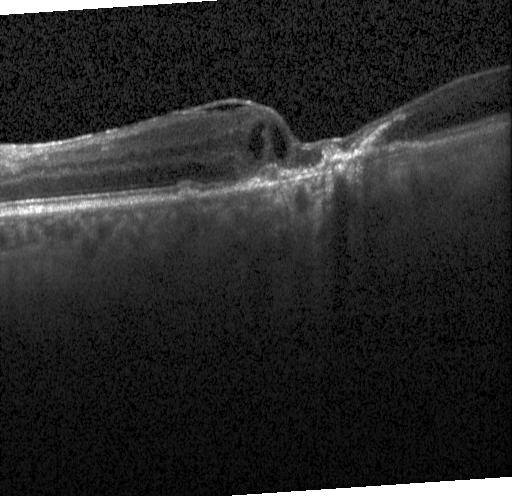

Heidelberg Spectralis · SD-OCT · retinal OCT cross-section — Finding: a choroidal neovascular membrane.